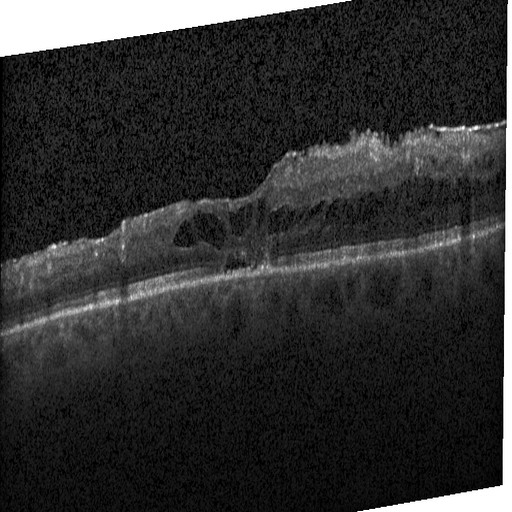
Horizontal scan through the fovea. SD-OCT. Heidelberg Spectralis OCT system. Retinal OCT B-scan — Macular OCT: DME.